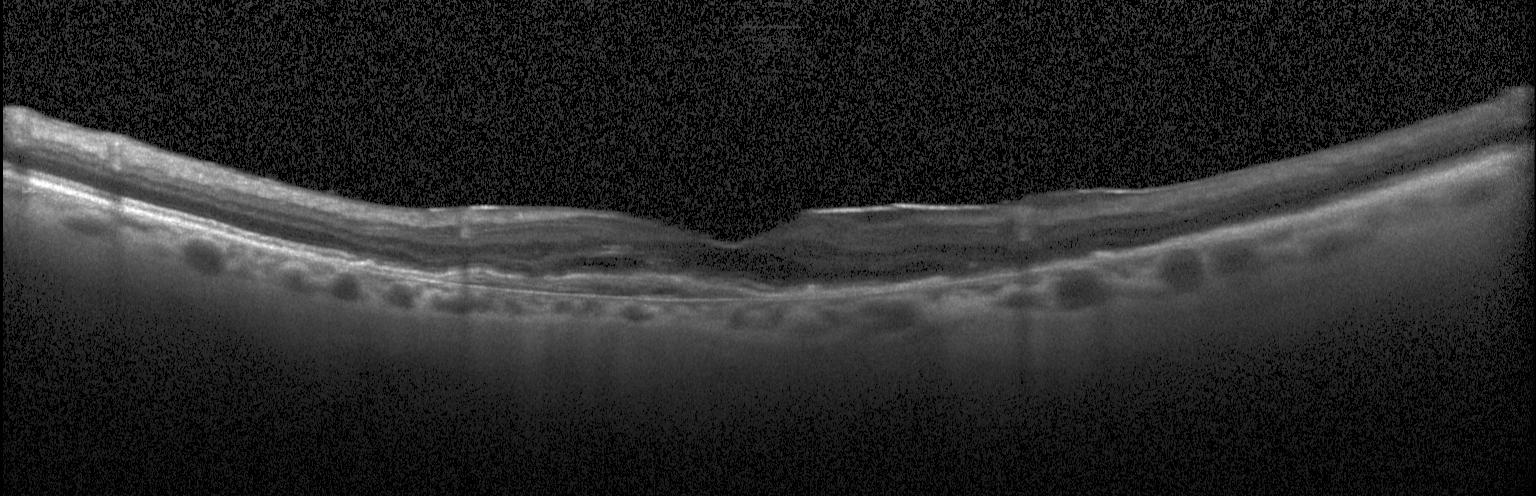
Macular OCT demonstrating a choroidal neovascular membrane.